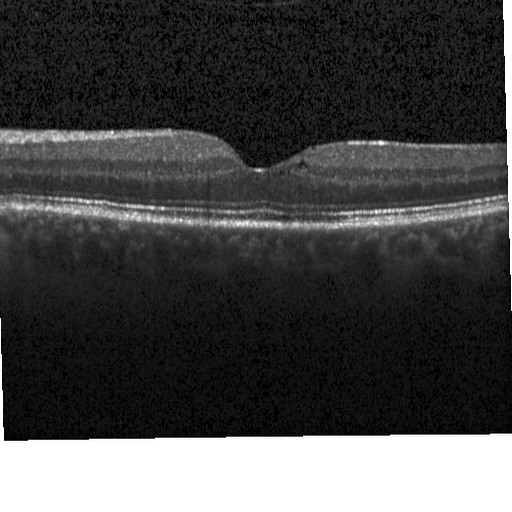

OCT line scan.
Assessment: DME.